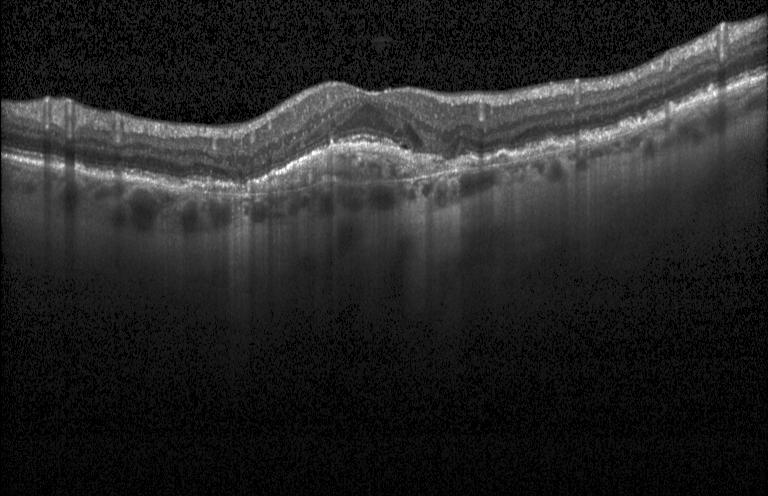 Macular scan · optical coherence tomography B-scan
Assessment: choroidal neovascularization.